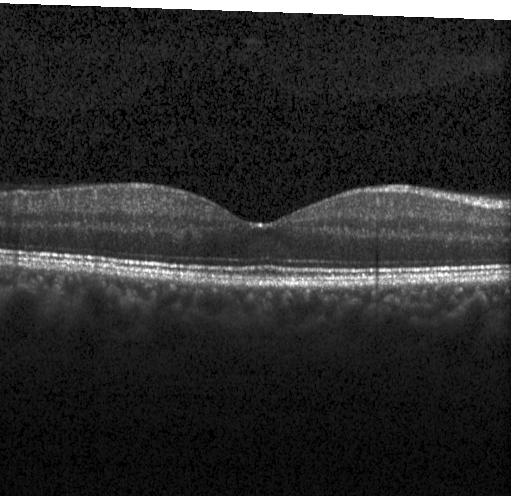

Horizontal scan through the fovea; OCT B-scan; acquired on a Heidelberg Spectralis — Dx: no choroidal neovascularization, diabetic macular edema, or drusen.